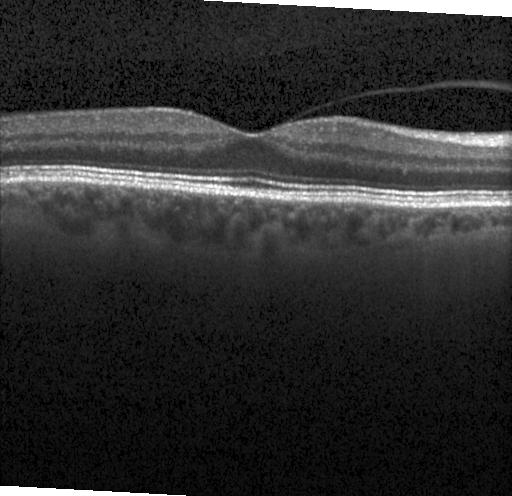 Macular scan; instrument: Heidelberg Spectralis; spectral-domain OCT; retinal OCT B-scan.
Finding: neither choroidal neovascularization, diabetic macular edema, nor drusen.